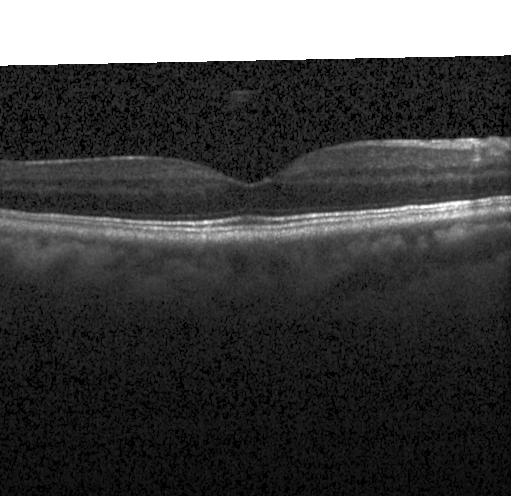

OCT B-scan.
Impression: no evidence of choroidal neovascularization, diabetic macular edema, or drusen.